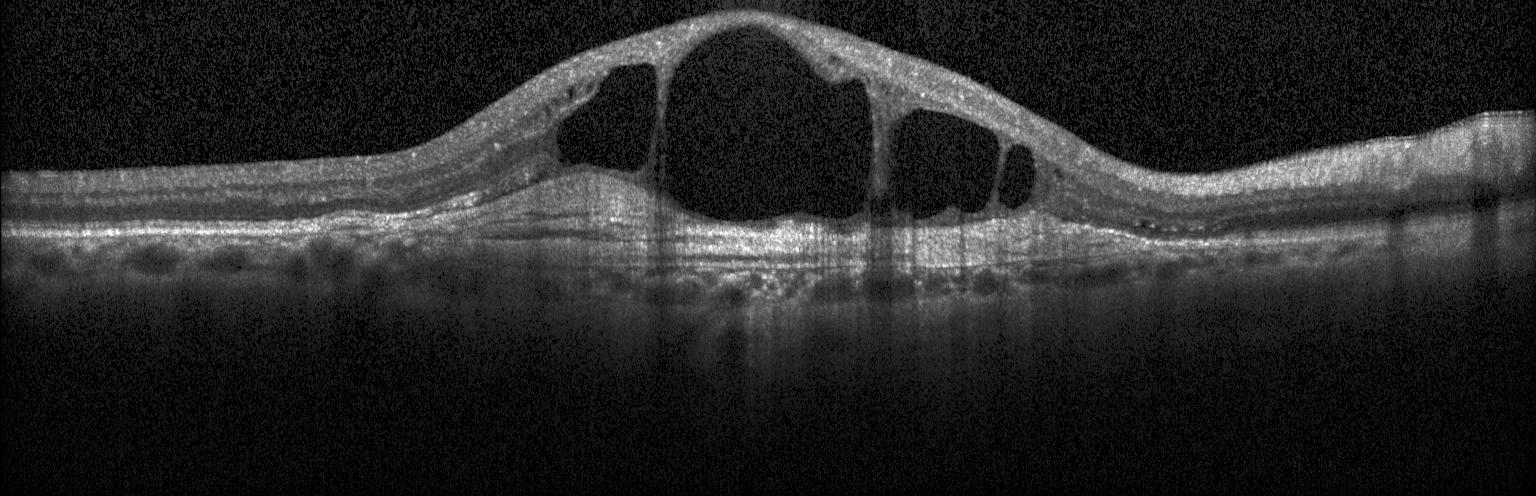 Optical coherence tomography B-scan; SD-OCT; macular scan; acquired on a Heidelberg Spectralis — Finding: CNV.